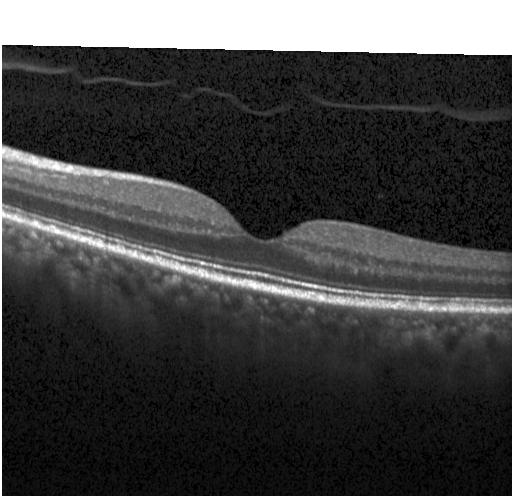
This B-scan demonstrates no choroidal neovascularization, diabetic macular edema, or drusen.